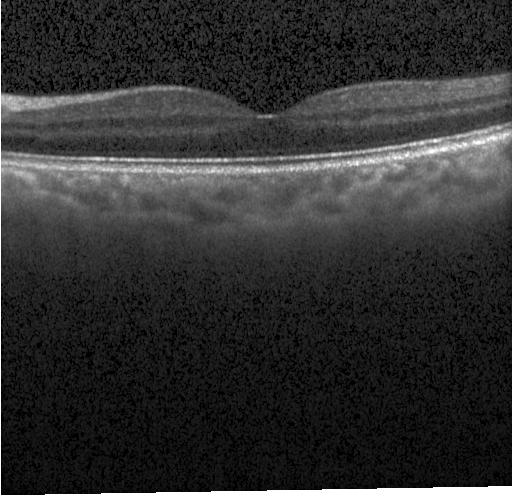 SD-OCT; optical coherence tomography scan; through the macula — Impression: no choroidal neovascularization, no diabetic macular edema, and no drusen.